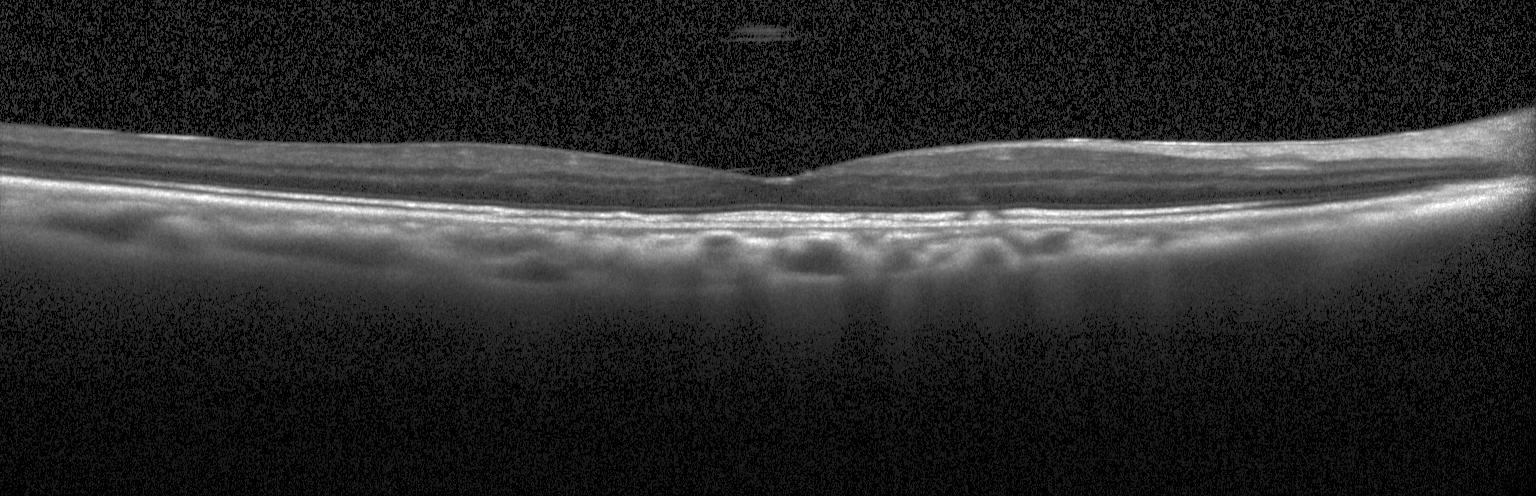 Through the macula, acquired on a Heidelberg Spectralis, OCT line scan. Diagnosis: no evidence of choroidal neovascularization, diabetic macular edema, or drusen.